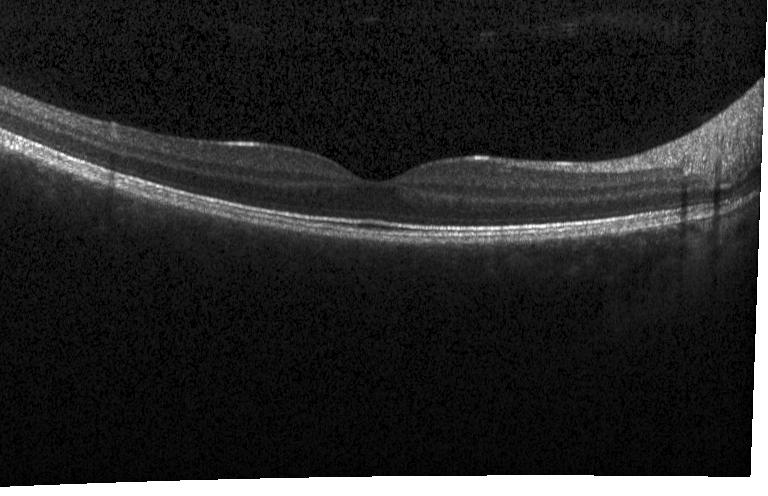 This B-scan demonstrates no CNV, no DME, and no drusen.